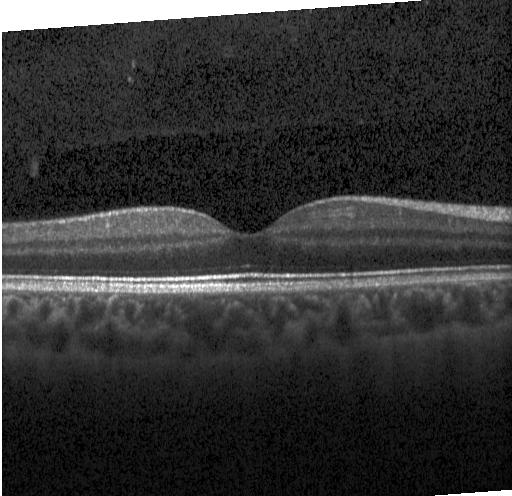

Assessment: no evidence of CNV, DME, or drusen.